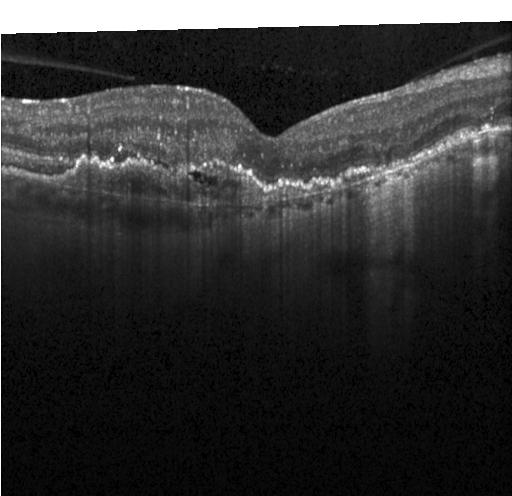
OCT finding: a choroidal neovascular membrane.